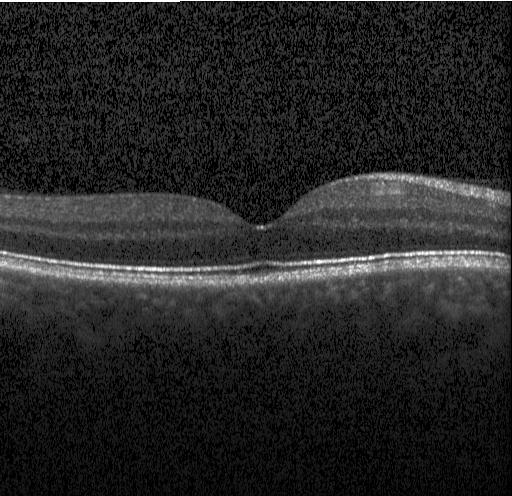
Retinal OCT B-scan — Diagnosis: no choroidal neovascularization, diabetic macular edema, or drusen.